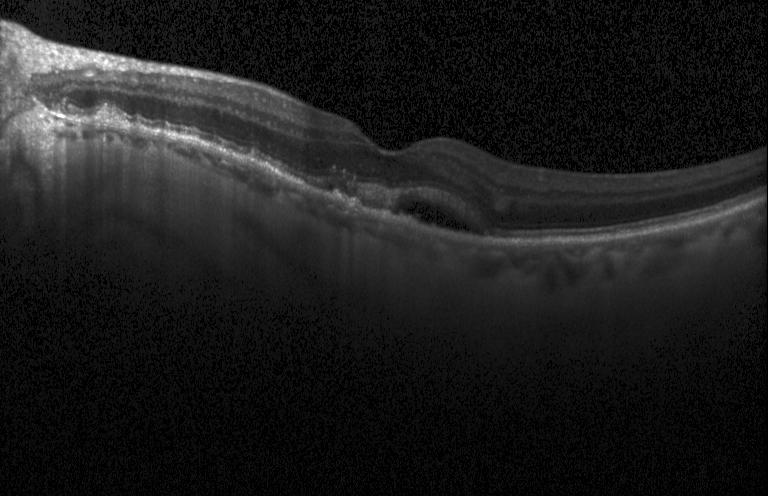 Optical coherence tomography B-scan, spectral-domain optical coherence tomography — OCT finding: a choroidal neovascular membrane.